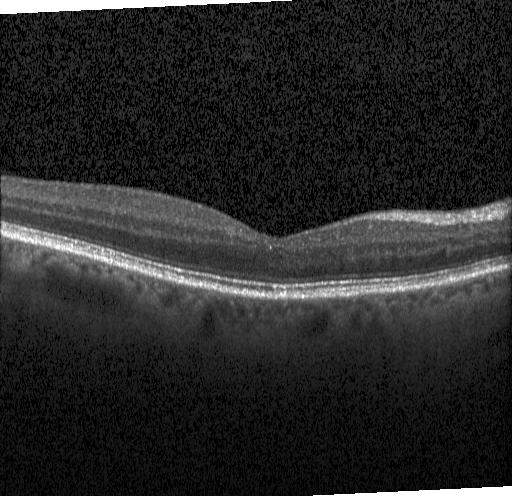

Acquired on a Heidelberg Spectralis · retinal OCT B-scan. Assessment: neither choroidal neovascularization, diabetic macular edema, nor drusen.